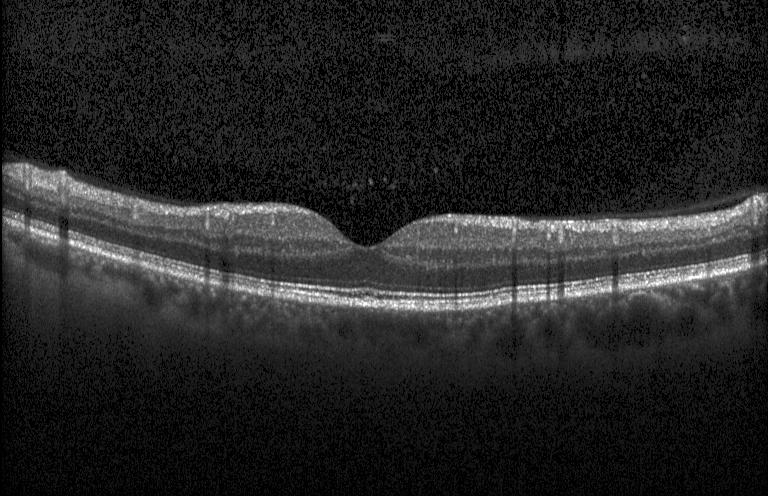
Optical coherence tomography scan
Finding: neither CNV, DME, nor drusen.